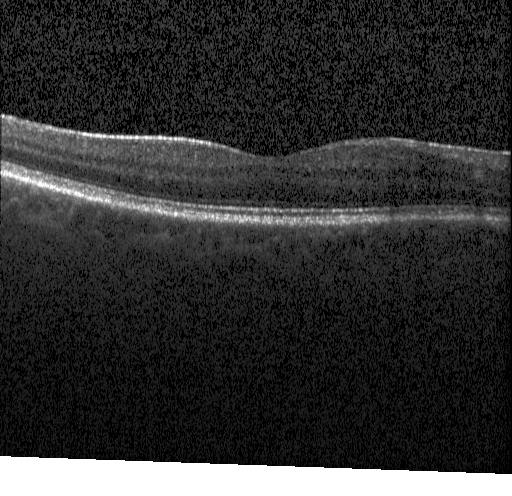
Optical coherence tomography scan. Acquired on a Heidelberg Spectralis. Macular scan. Spectral-domain optical coherence tomography.
Macular OCT: neither choroidal neovascularization, diabetic macular edema, nor drusen.